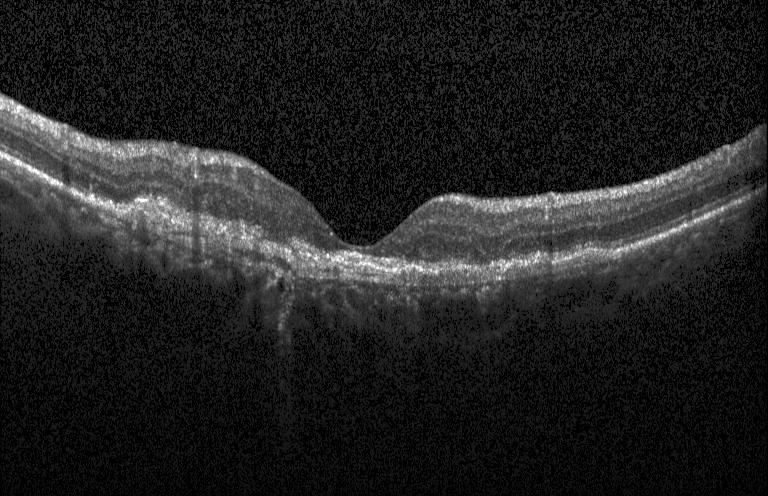
Dx: a choroidal neovascular membrane.